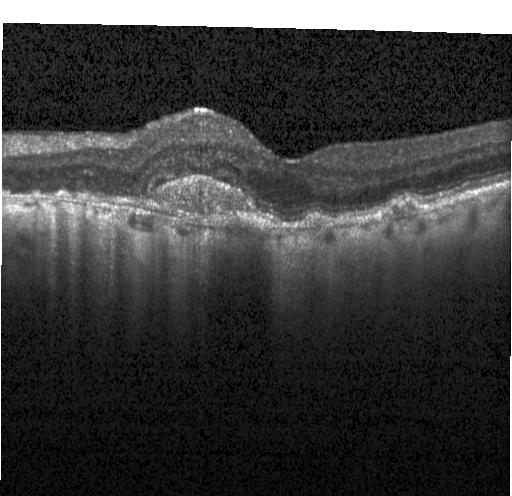
Macular scan; retinal OCT cross-section; instrument: Heidelberg Spectralis; SD-OCT. Finding: choroidal neovascularization (CNV).